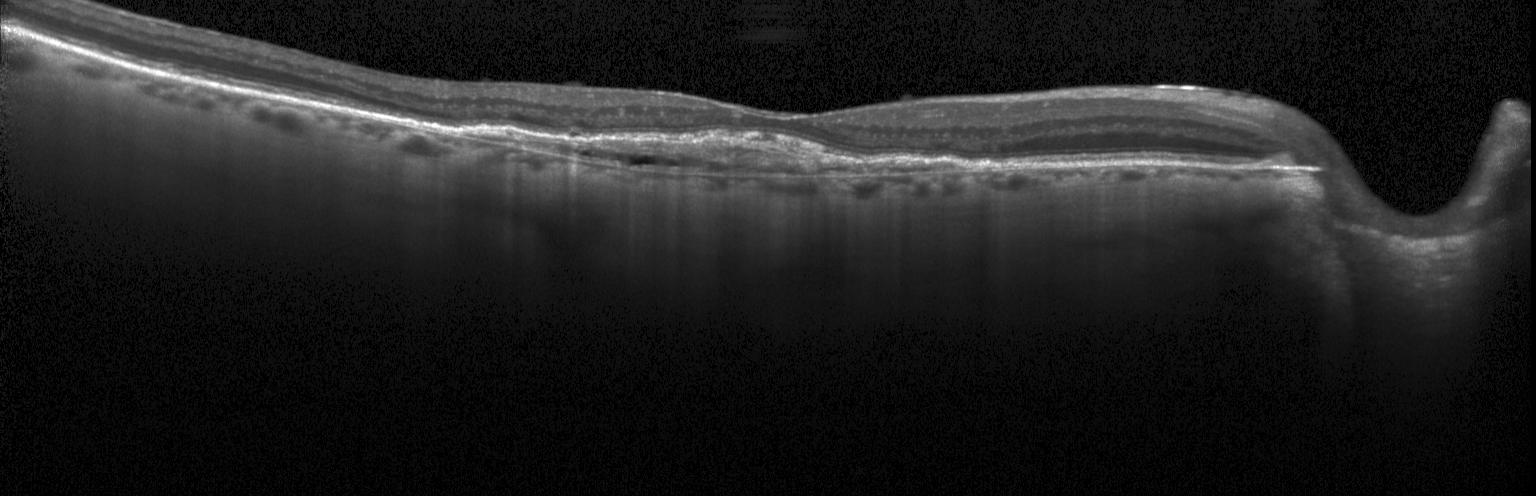
Optical coherence tomography scan; SD-OCT; instrument: Heidelberg Spectralis; centered on the fovea. The scan shows choroidal neovascularization (CNV).